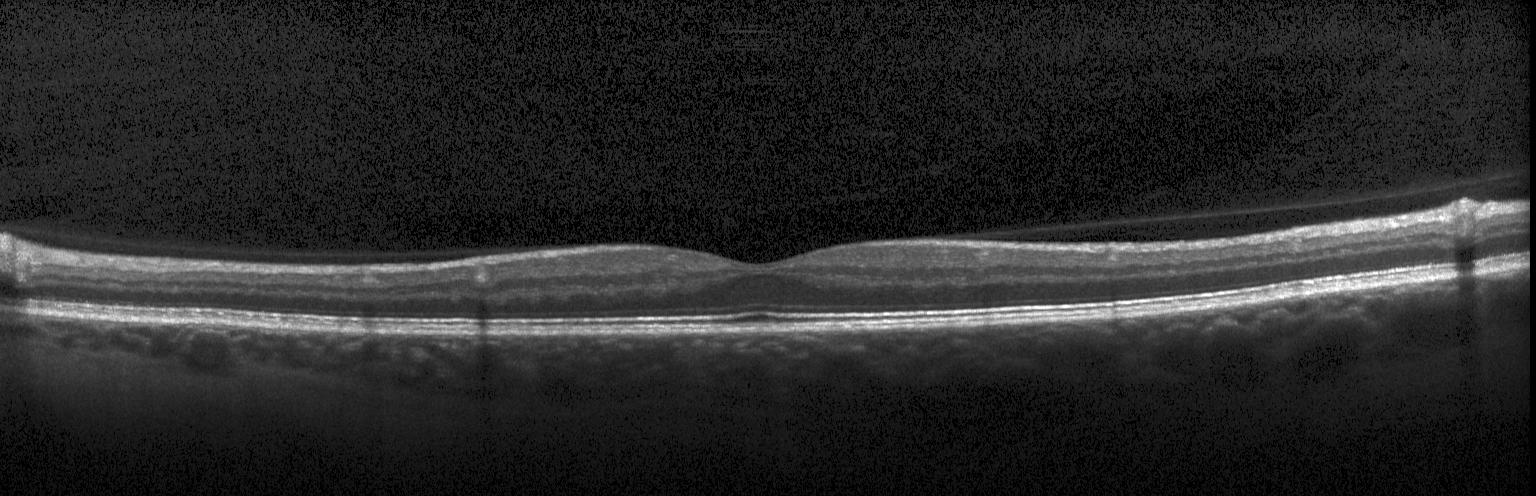
Optical coherence tomography B-scan. Heidelberg Spectralis OCT system — The scan shows neither choroidal neovascularization, diabetic macular edema, nor drusen.